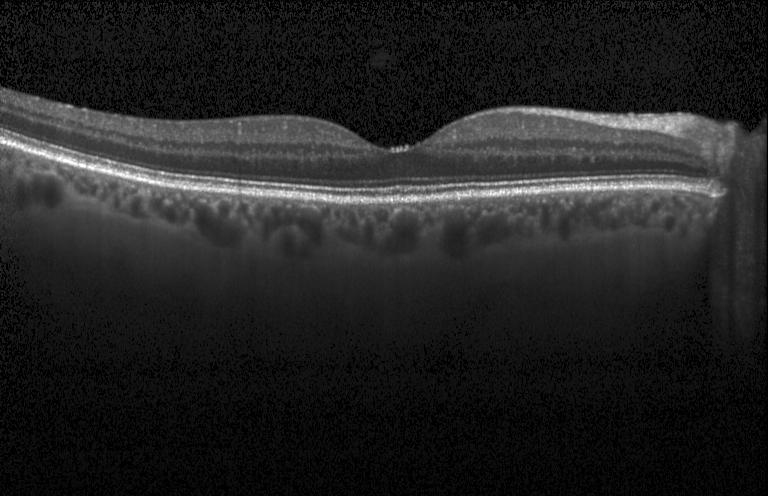 Spectral-domain optical coherence tomography. Fovea-centered. Optical coherence tomography B-scan. Instrument: Heidelberg Spectralis — Diagnosis: no choroidal neovascularization, no diabetic macular edema, and no drusen.